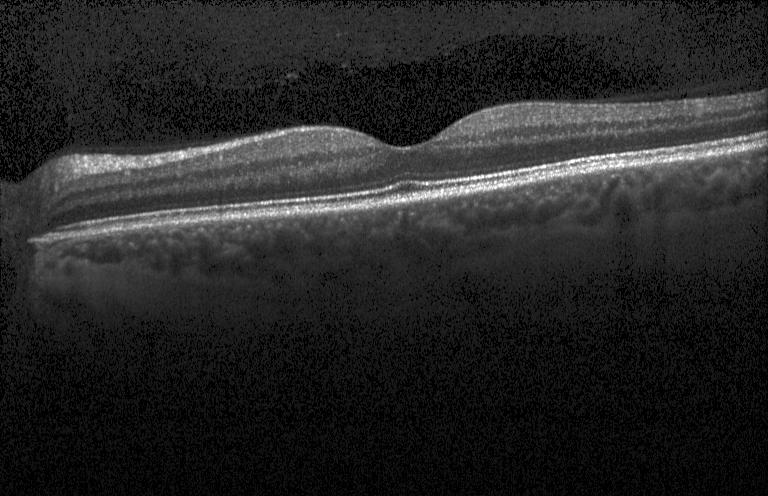

SD-OCT. Heidelberg Spectralis. Retinal OCT B-scan — Assessment: no choroidal neovascularization, no diabetic macular edema, and no drusen.